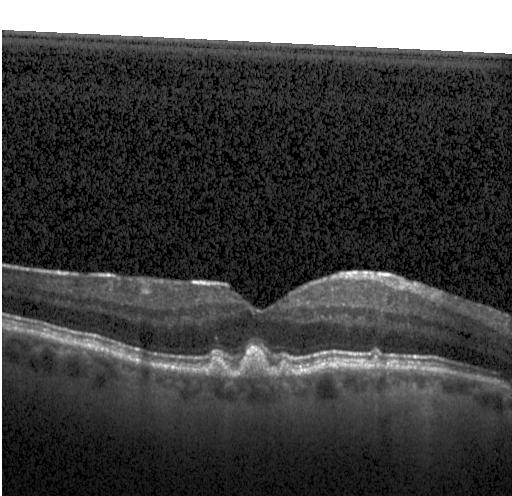

Impression: multiple drusen.